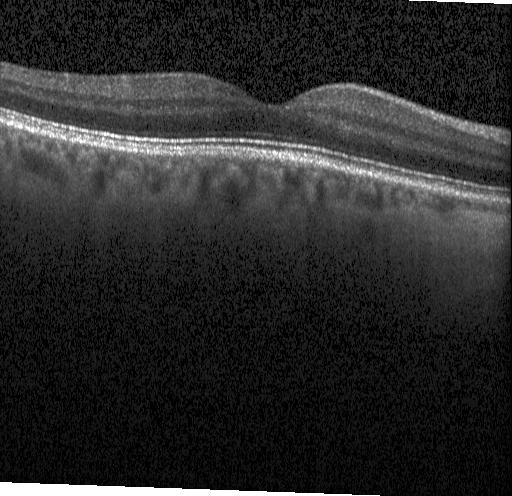

Diagnosis: no evidence of choroidal neovascularization, diabetic macular edema, or drusen.